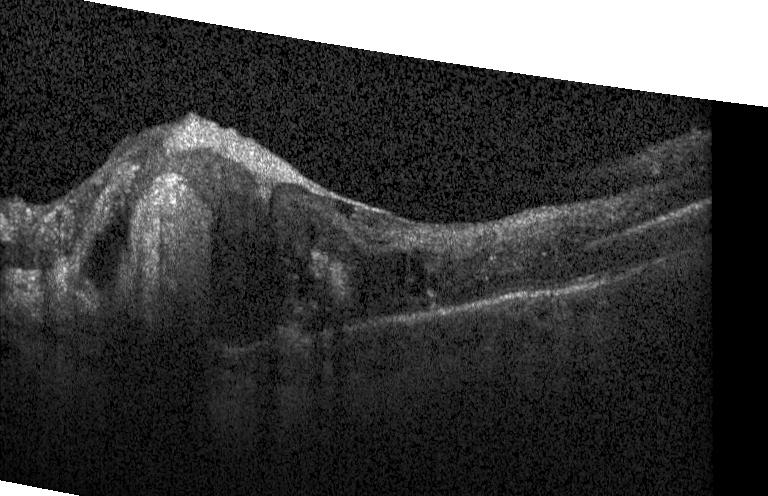

Heidelberg Spectralis OCT system · through the macula · optical coherence tomography scan. Finding: a choroidal neovascular membrane.